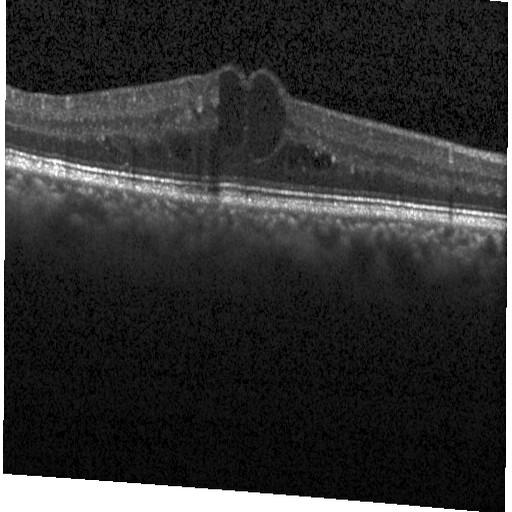
Optical coherence tomography scan.
Impression: diabetic macular edema.